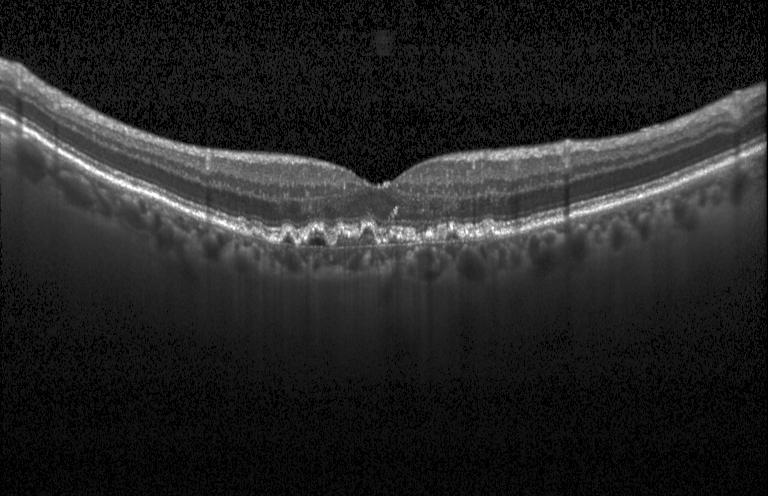 Centered on the fovea, acquired on a Heidelberg Spectralis, SD-OCT, retinal OCT cross-section. Macular OCT: drusen.